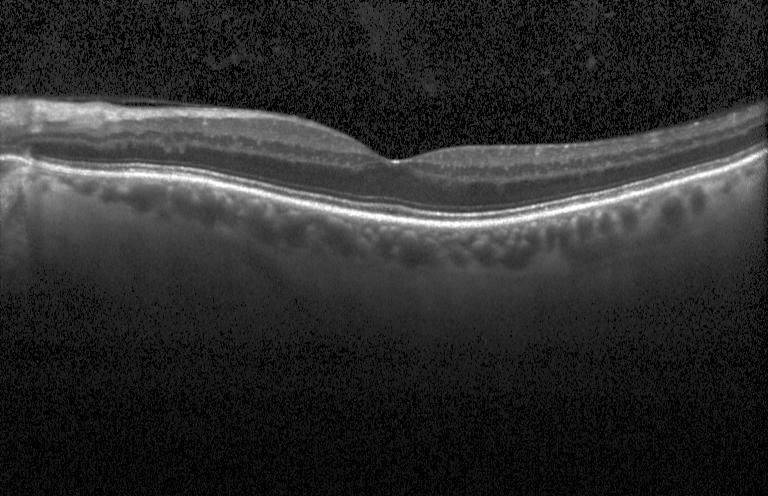 Diagnosis: no CNV, no DME, and no drusen.